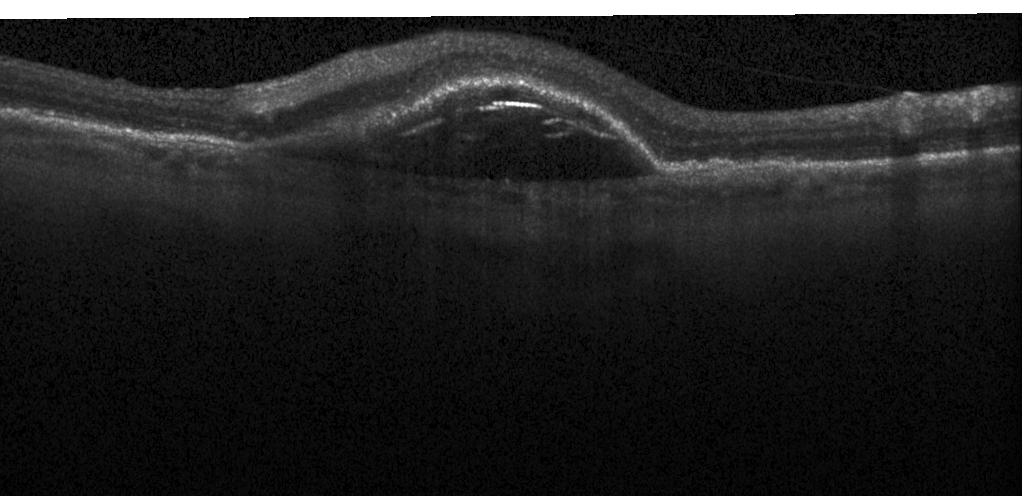
Retinal OCT B-scan; Heidelberg Spectralis OCT system — A choroidal neovascular membrane.